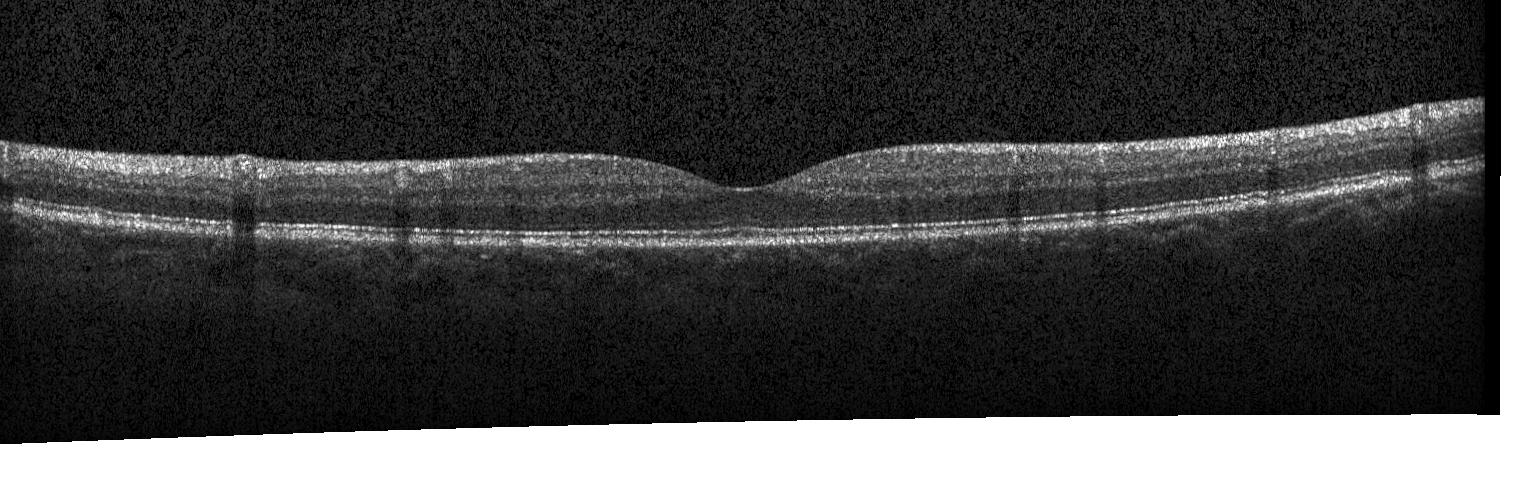

Neither choroidal neovascularization, diabetic macular edema, nor drusen.